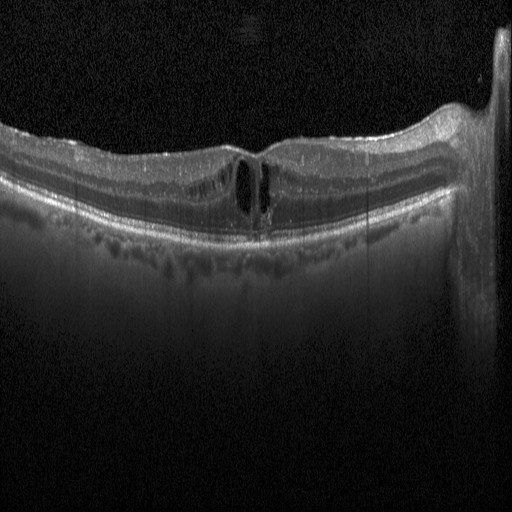
Retinal OCT B-scan
This B-scan demonstrates diabetic macular edema (DME).